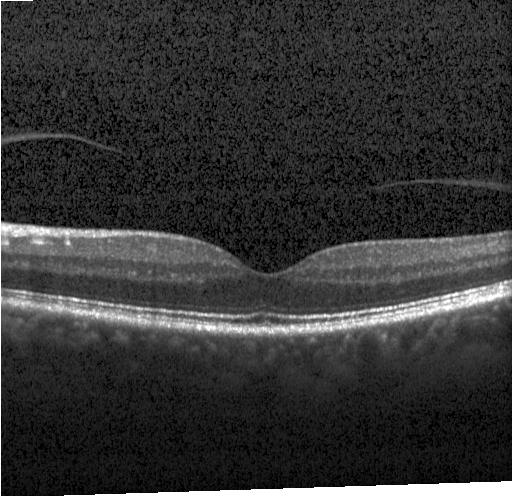

Spectral-domain optical coherence tomography. Acquired on a Heidelberg Spectralis. Centered on the fovea. OCT line scan. Finding: no evidence of CNV, DME, or drusen.